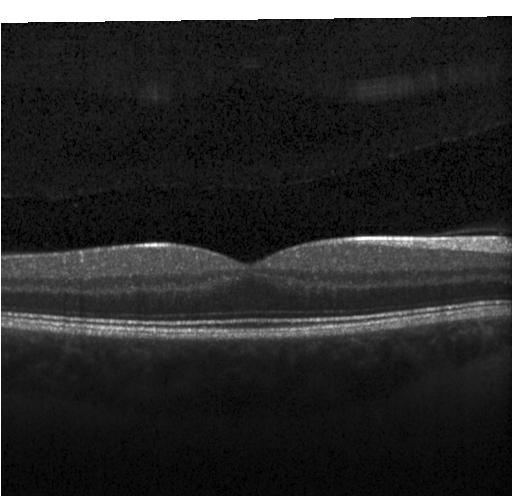
OCT finding: no evidence of CNV, DME, or drusen.